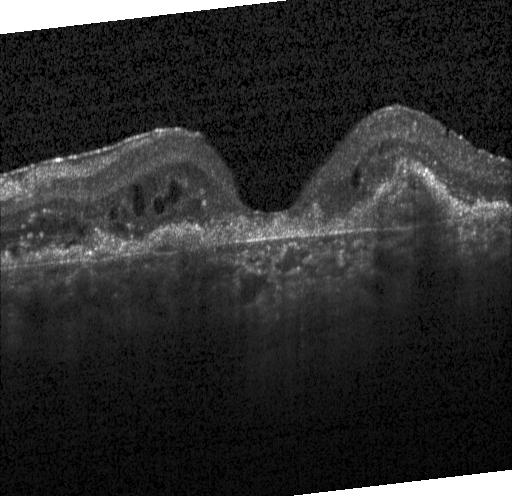 OCT B-scan showing choroidal neovascularization (CNV).